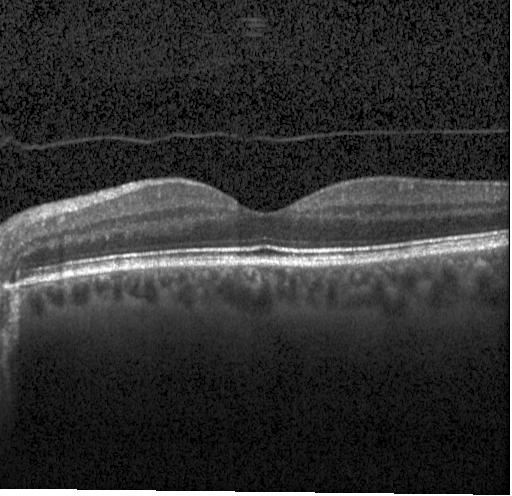
SD-OCT · retinal OCT B-scan · centered on the fovea — Assessment: neither choroidal neovascularization, diabetic macular edema, nor drusen.